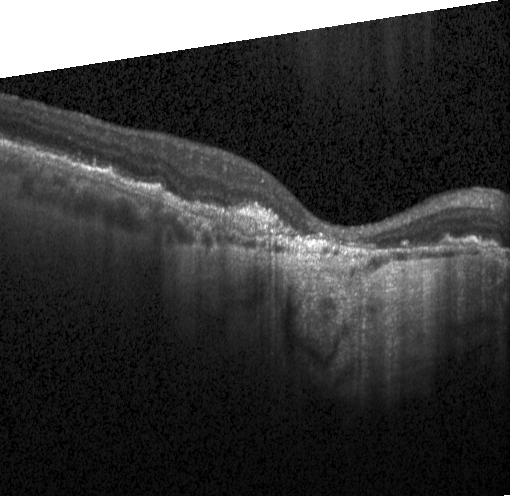 OCT scan showing a choroidal neovascular membrane.